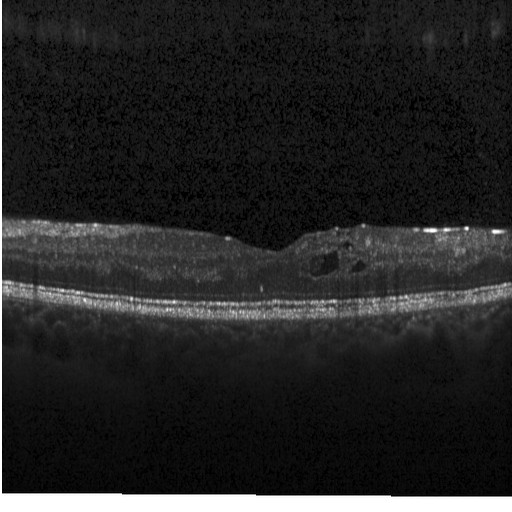
Acquired on a Heidelberg Spectralis. Optical coherence tomography B-scan. Fovea-centered.
This B-scan demonstrates DME.